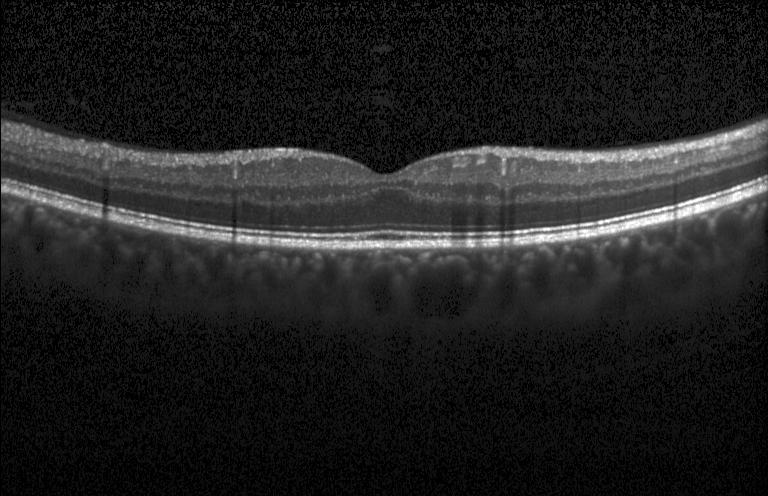

Spectral-domain OCT, optical coherence tomography scan, Heidelberg Spectralis OCT system.
Diagnosis: neither choroidal neovascularization, diabetic macular edema, nor drusen.